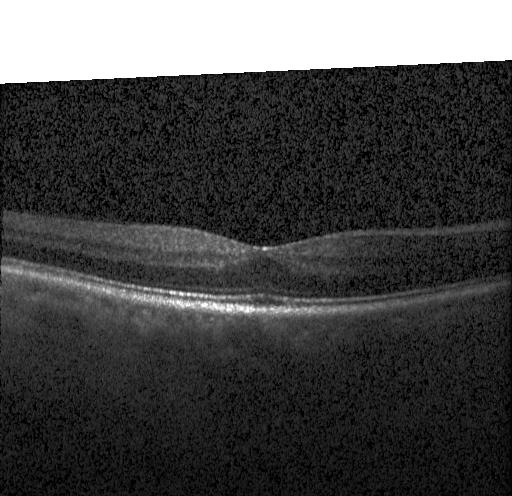

Macular OCT: no choroidal neovascularization, diabetic macular edema, or drusen.